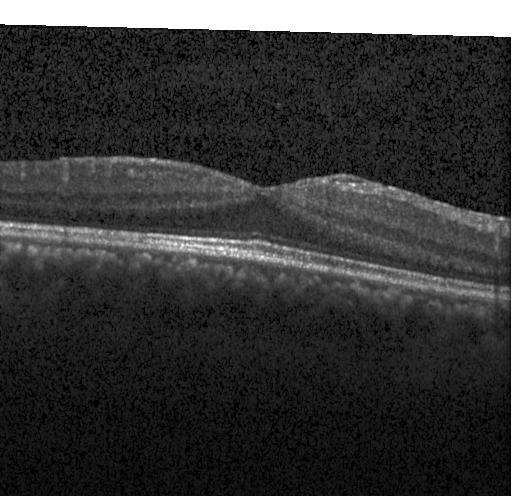

Instrument: Heidelberg Spectralis · SD-OCT · OCT line scan. Finding: no choroidal neovascularization, diabetic macular edema, or drusen.